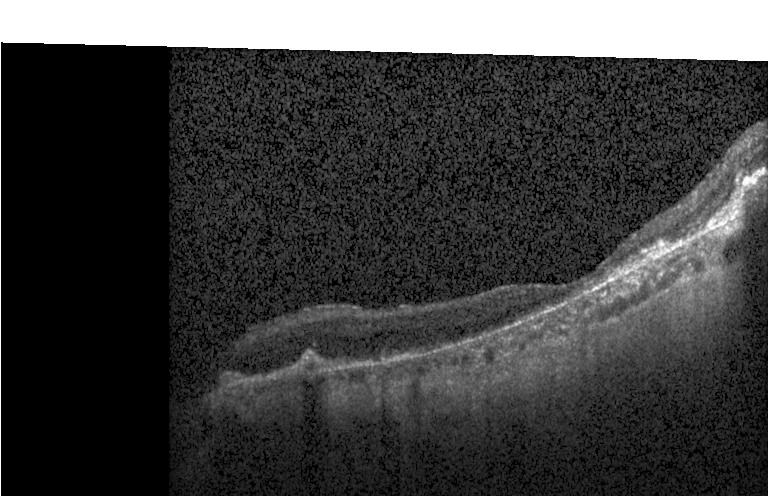

Dx: a choroidal neovascular membrane.